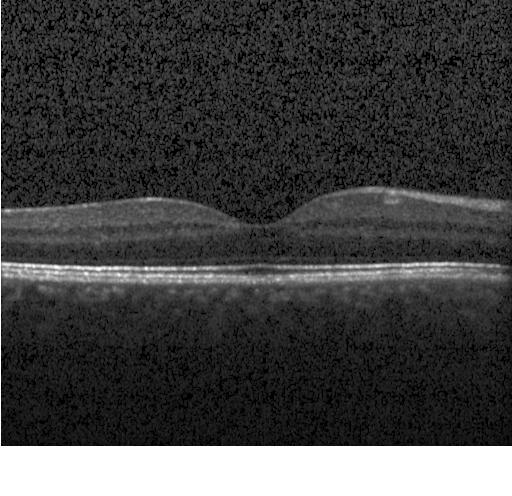

Macular OCT: no evidence of choroidal neovascularization, diabetic macular edema, or drusen.